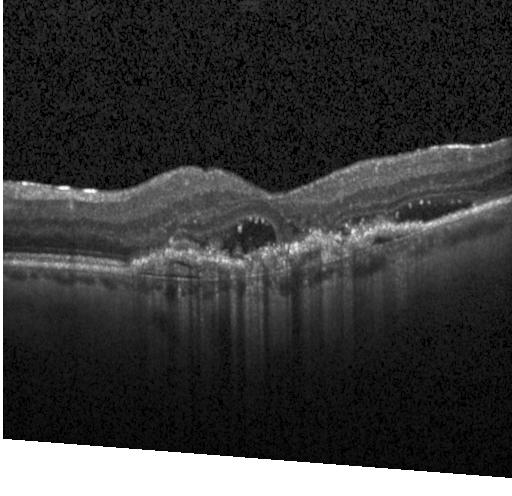
Heidelberg Spectralis. OCT line scan. Diagnosis: a choroidal neovascular membrane.